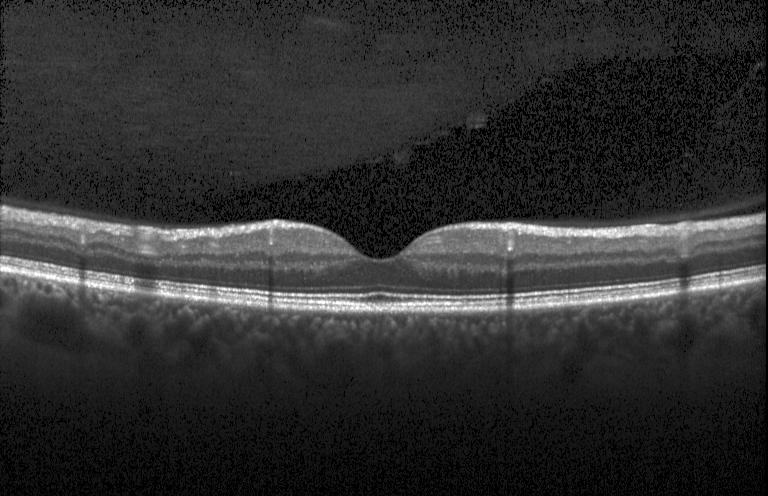

Spectral-domain optical coherence tomography. Optical coherence tomography scan. Centered on the fovea
Impression: no evidence of choroidal neovascularization, diabetic macular edema, or drusen.